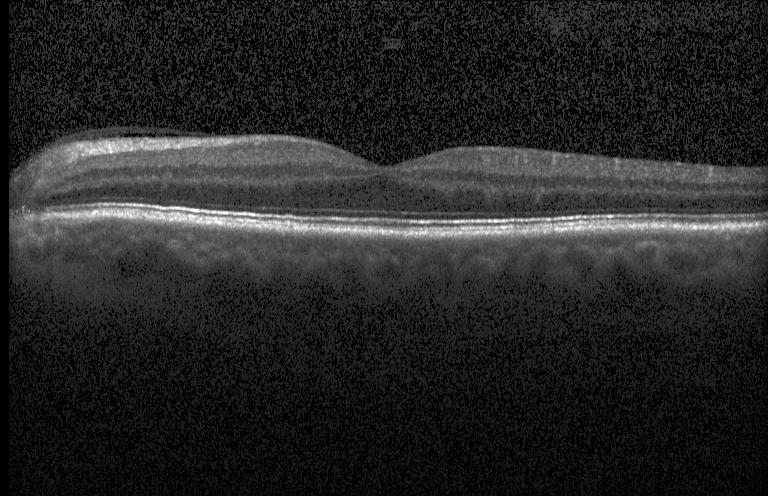 Spectral-domain optical coherence tomography; retinal OCT cross-section; centered on the fovea. Dx: no choroidal neovascularization, no diabetic macular edema, and no drusen.